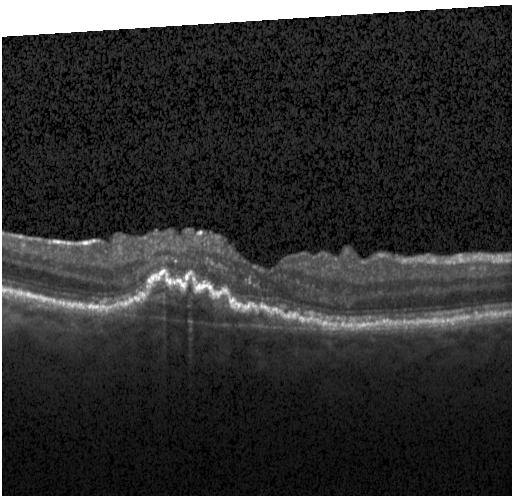

Macular OCT demonstrating a choroidal neovascular membrane.